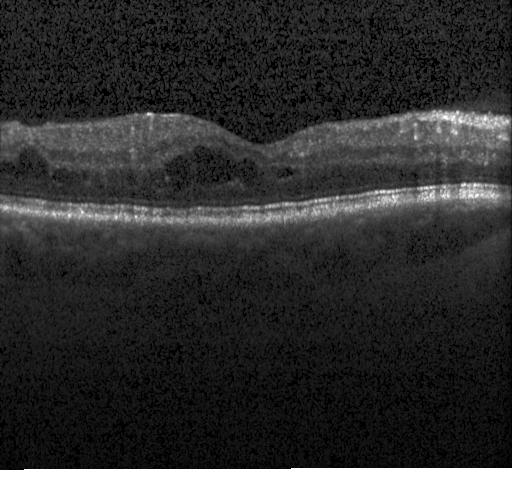 OCT scan showing diabetic macular edema.